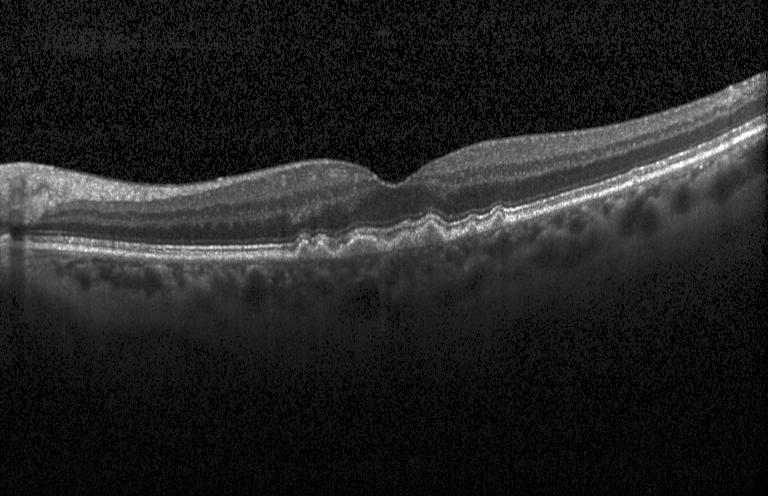

Macular OCT: sub-RPE drusenoid deposits.